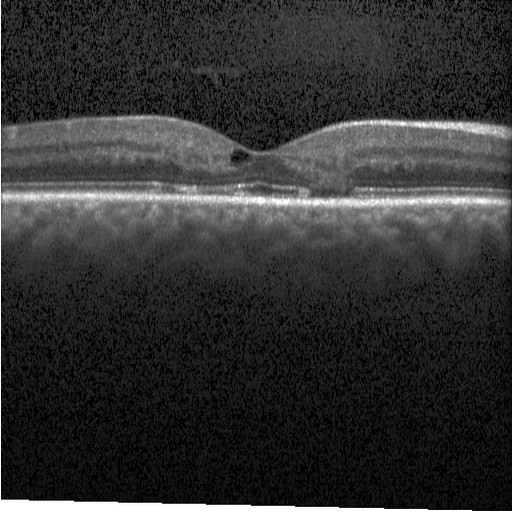

Macular OCT: diabetic macular edema.